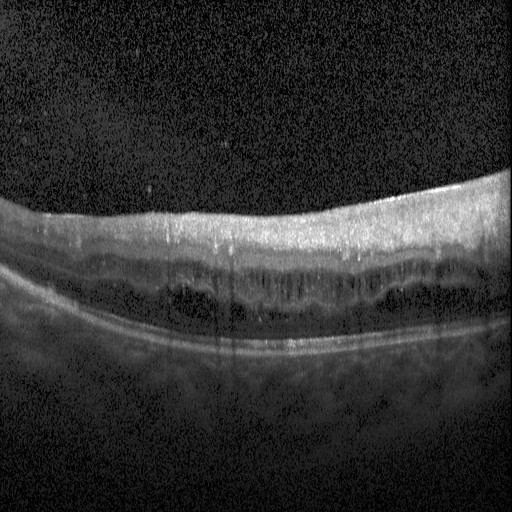 Finding: diabetic macular edema (DME).